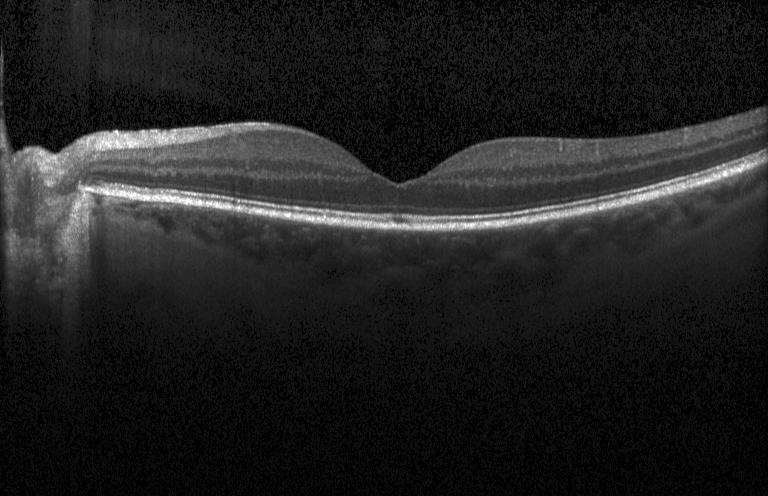 Impression: neither choroidal neovascularization, diabetic macular edema, nor drusen.